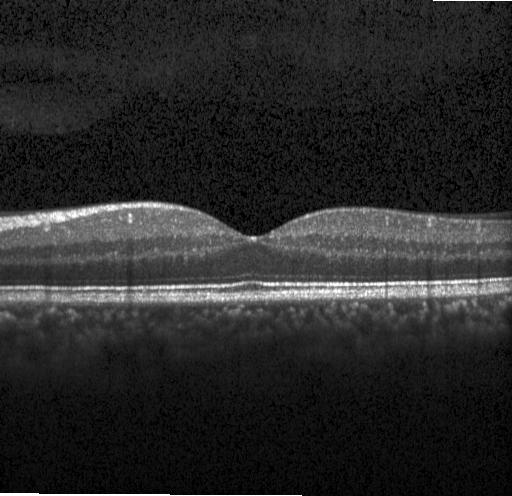
Optical coherence tomography B-scan. The scan shows neither choroidal neovascularization, diabetic macular edema, nor drusen.